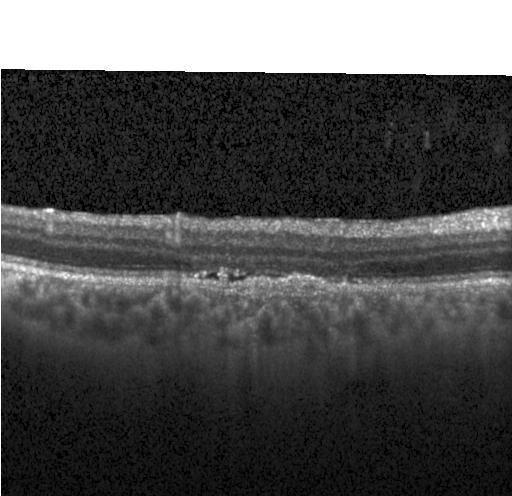 Optical coherence tomography scan. Through the macula. Spectral-domain optical coherence tomography. Acquired on a Heidelberg Spectralis
Finding: a choroidal neovascular membrane.